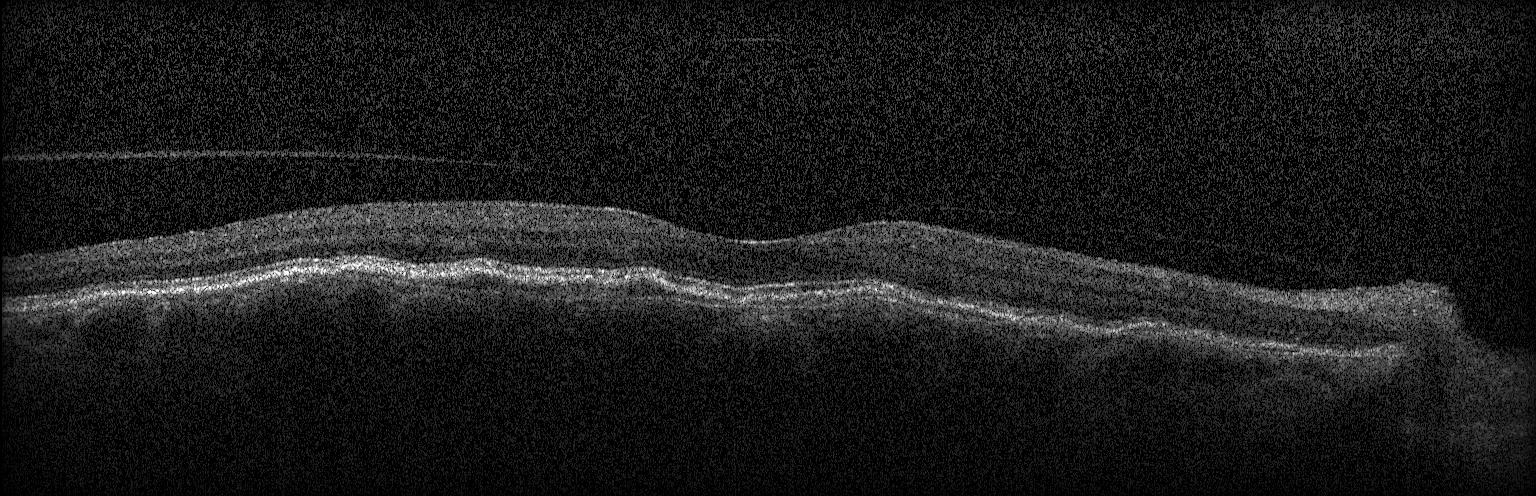
Impression: a choroidal neovascular membrane.